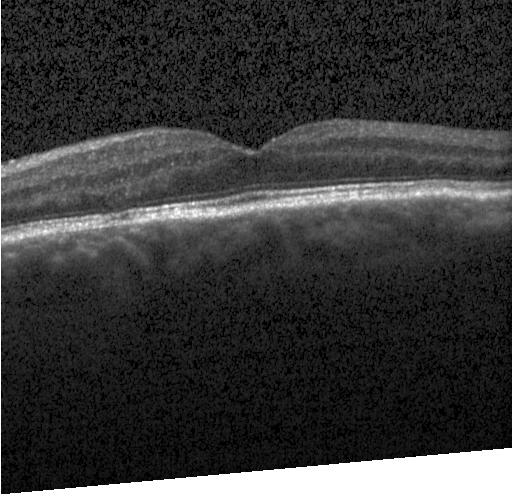

Retinal OCT B-scan. Spectral-domain OCT. Heidelberg Spectralis. Macular scan. Finding: no choroidal neovascularization, no diabetic macular edema, and no drusen.